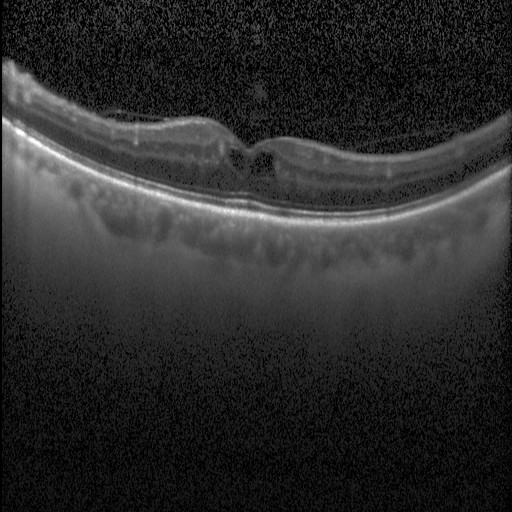 Impression: diabetic macular edema.